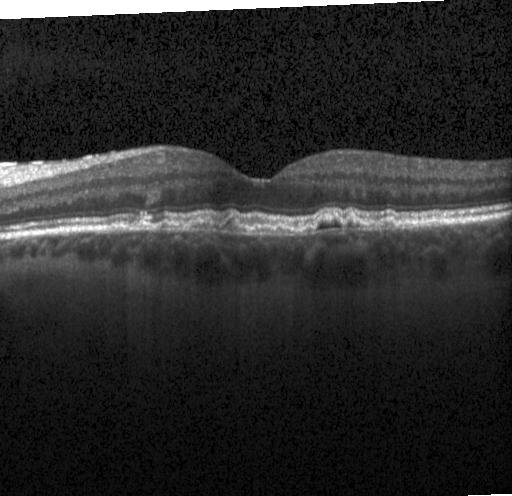 Retinal OCT cross-section · horizontal scan through the fovea · instrument: Heidelberg Spectralis · spectral-domain OCT.
Finding: sub-RPE drusenoid deposits.